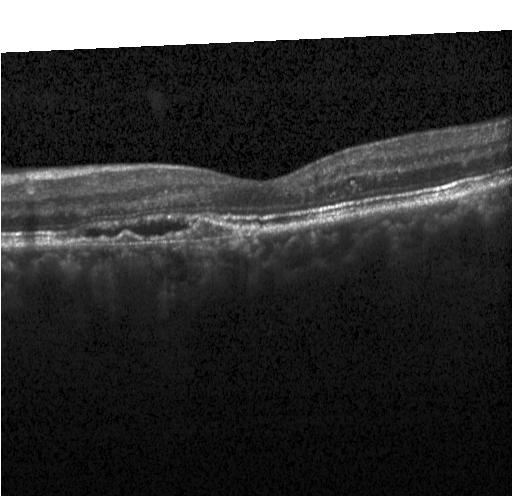
Dx: CNV.